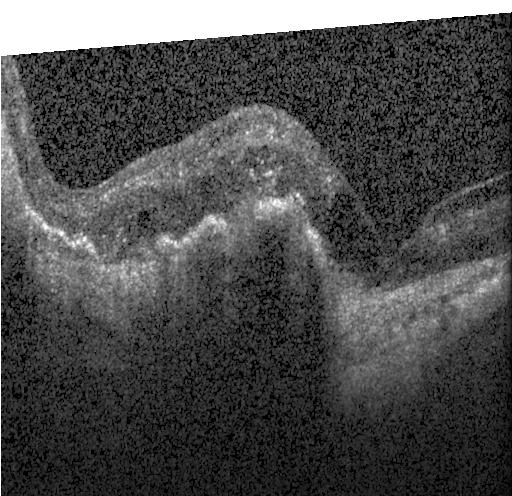

OCT line scan. Acquired on a Heidelberg Spectralis. Macular scan.
Impression: CNV.